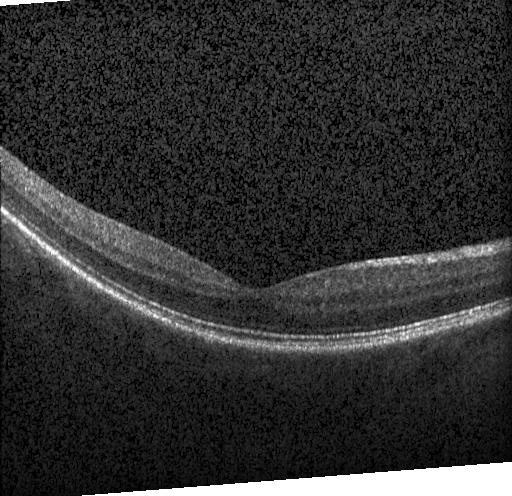 Optical coherence tomography B-scan
No choroidal neovascularization, diabetic macular edema, or drusen.